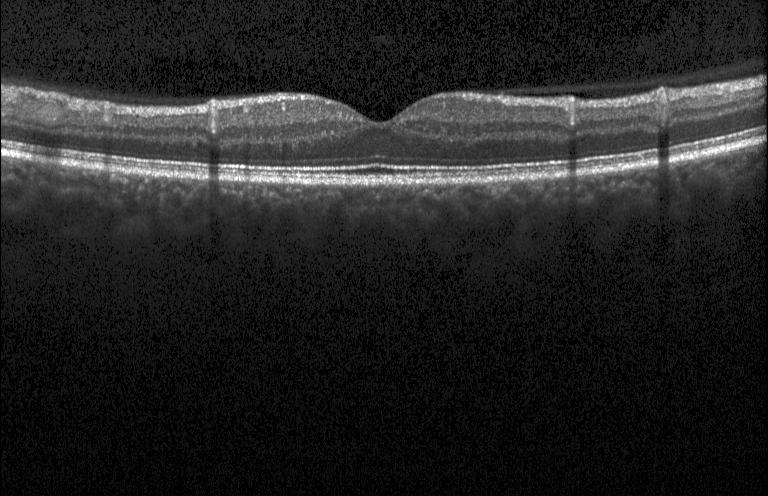

The scan shows no CNV, DME, or drusen.